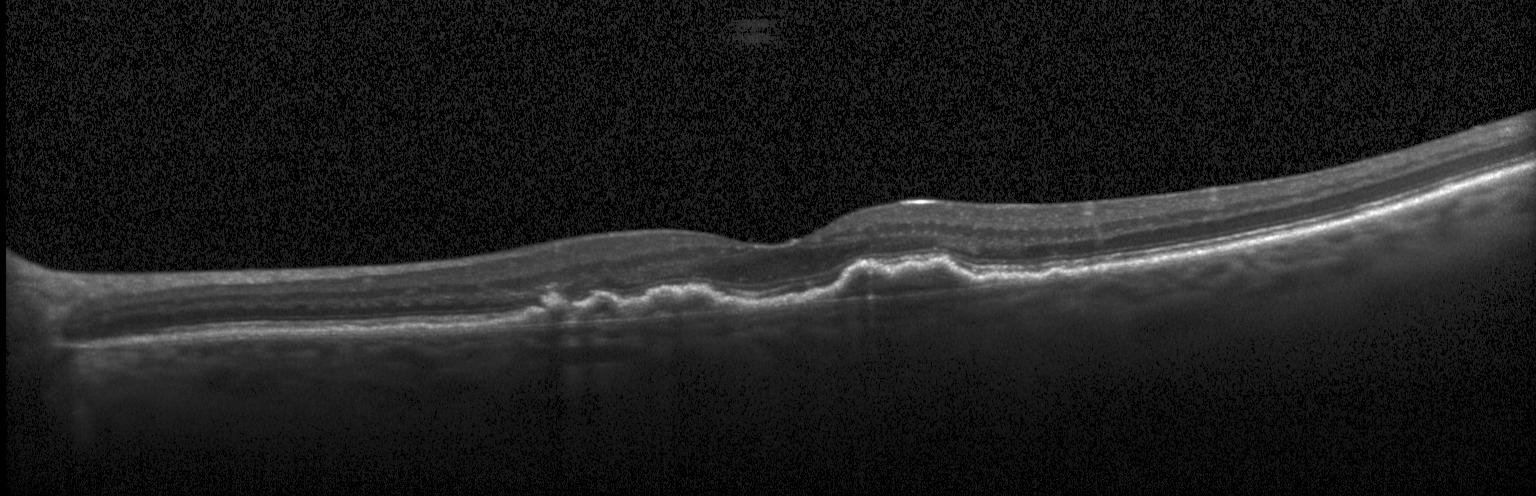
Heidelberg Spectralis OCT system · fovea-centered · retinal OCT cross-section · spectral-domain OCT.
Impression: choroidal neovascularization (CNV).